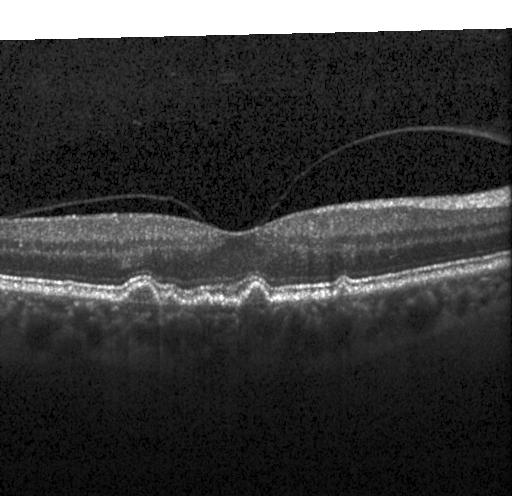

Optical coherence tomography B-scan; spectral-domain optical coherence tomography
Multiple drusen.